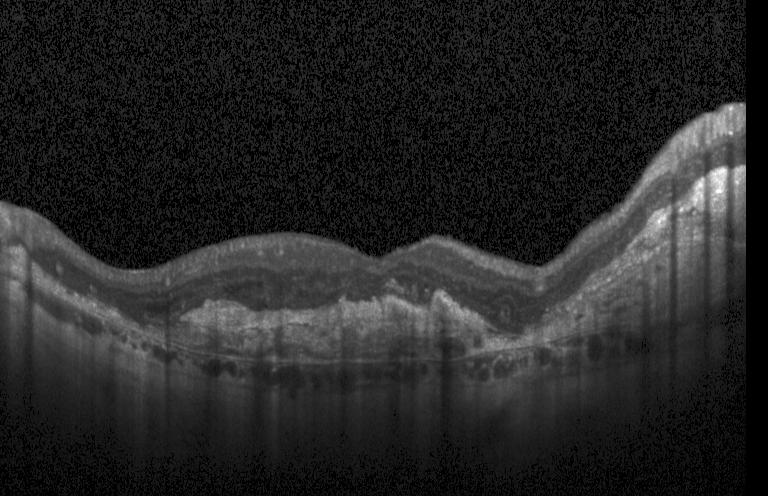
Optical coherence tomography B-scan. Heidelberg Spectralis OCT system.
Macular OCT: a choroidal neovascular membrane.